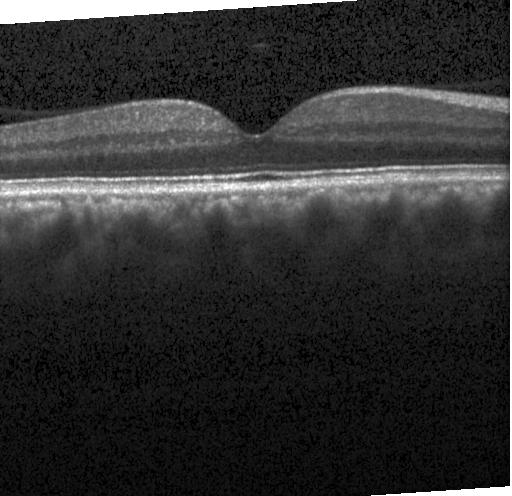

Optical coherence tomography B-scan; spectral-domain optical coherence tomography; centered on the fovea.
Diagnosis: no choroidal neovascularization, diabetic macular edema, or drusen.